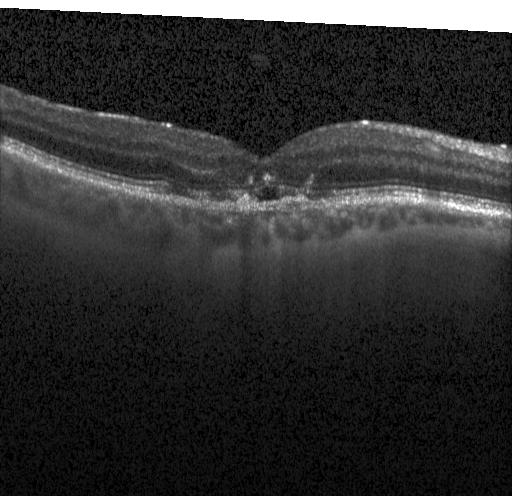

OCT finding: a choroidal neovascular membrane.